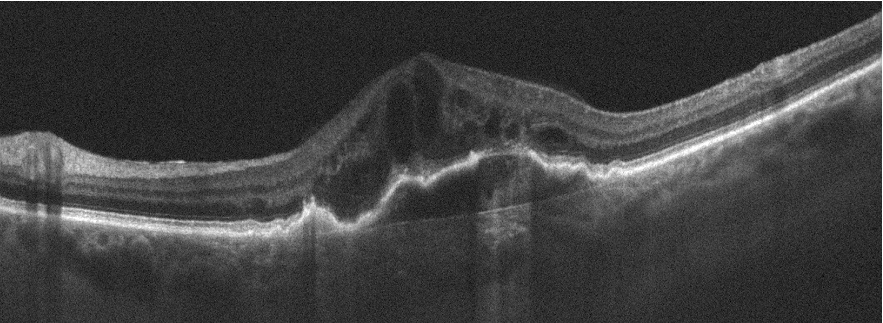
Optical coherence tomography B-scan.
Impression: AMD.